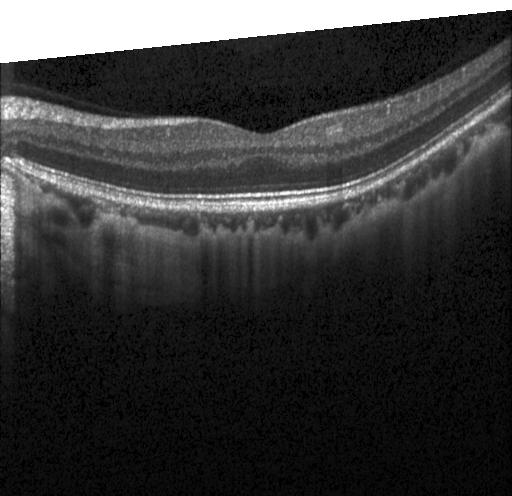

Spectral-domain optical coherence tomography, retinal OCT cross-section. The scan shows no evidence of choroidal neovascularization, diabetic macular edema, or drusen.